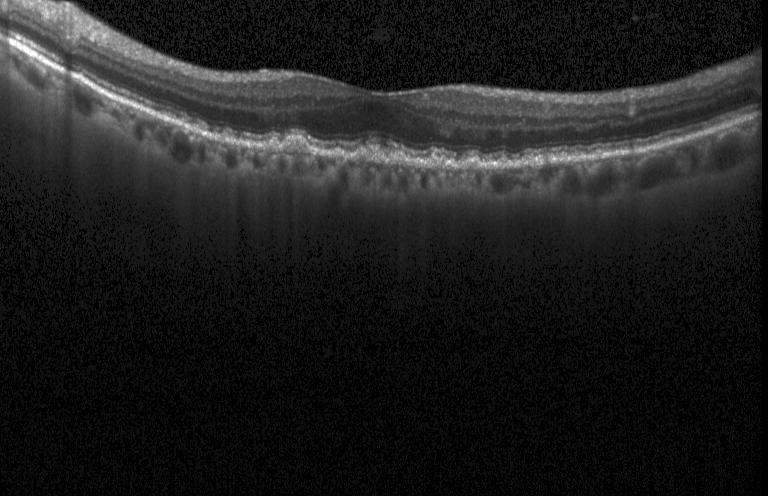
Optical coherence tomography scan; centered on the fovea; SD-OCT; instrument: Heidelberg Spectralis — Dx: multiple drusen.